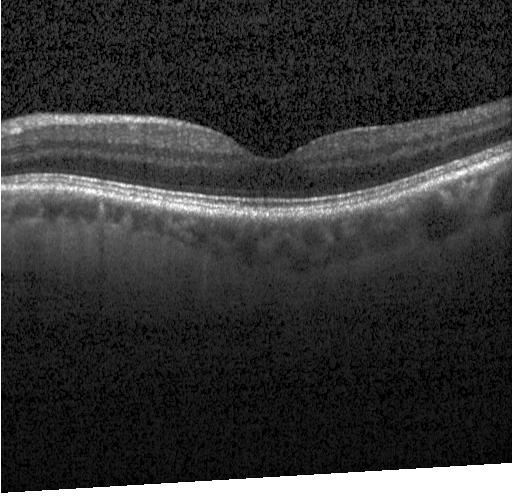 Optical coherence tomography scan. Diagnosis: no evidence of choroidal neovascularization, diabetic macular edema, or drusen.